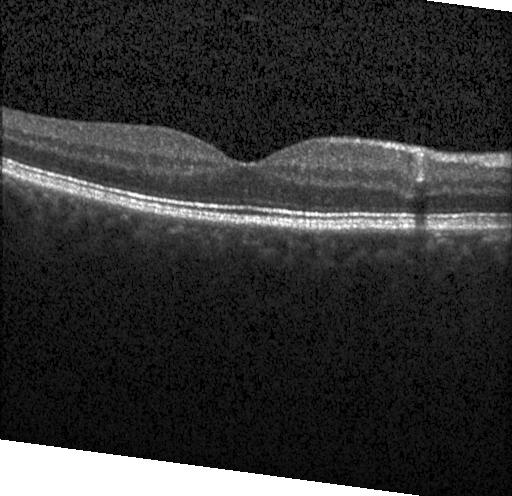 Retinal OCT B-scan; SD-OCT; Heidelberg Spectralis OCT system; horizontal scan through the fovea
Assessment: no choroidal neovascularization, diabetic macular edema, or drusen.